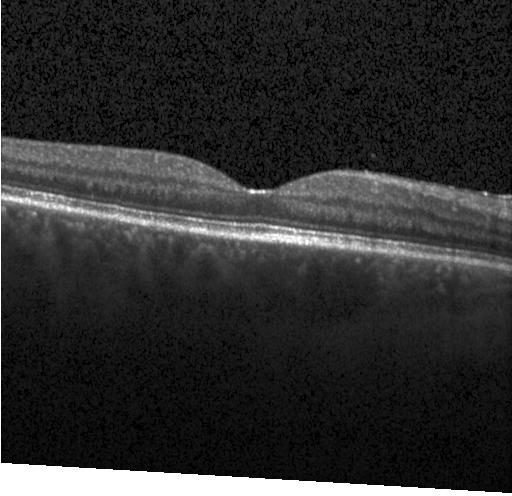
Retinal OCT B-scan
Finding: no choroidal neovascularization, no diabetic macular edema, and no drusen.